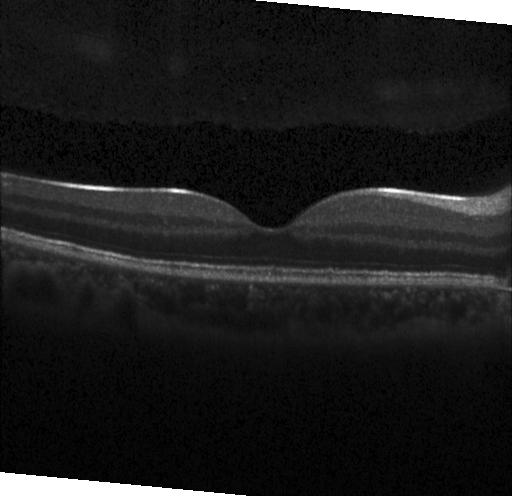

Impression: no evidence of choroidal neovascularization, diabetic macular edema, or drusen.